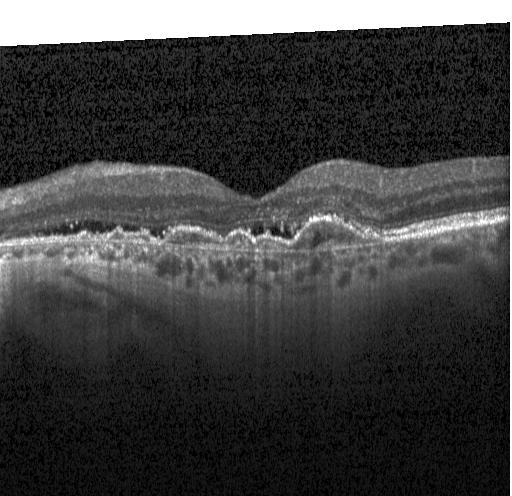
Macular OCT: a choroidal neovascular membrane.